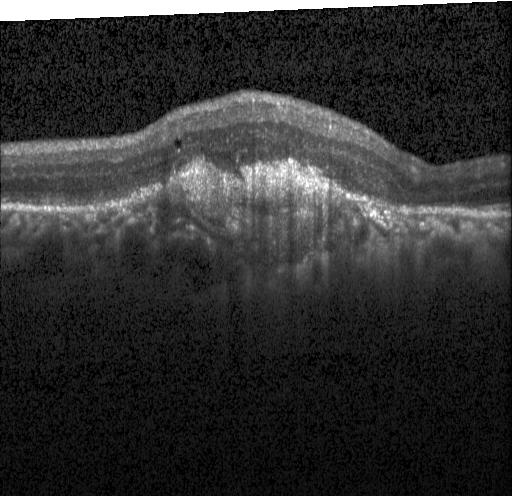 Assessment: a choroidal neovascular membrane.